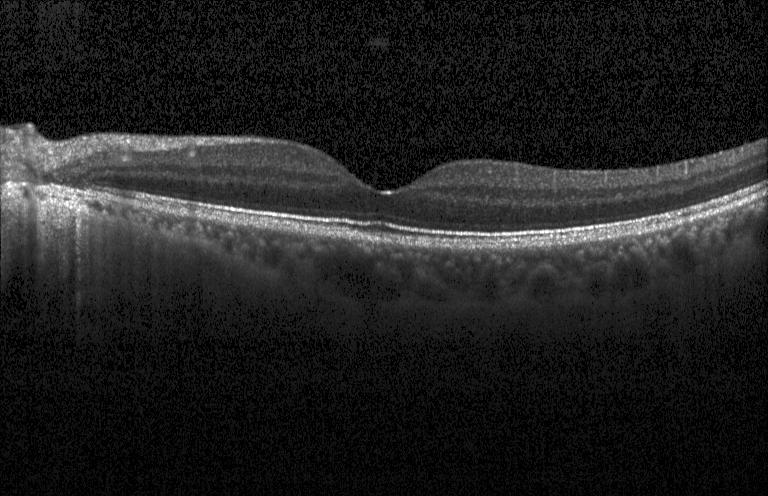
Optical coherence tomography B-scan — This B-scan demonstrates neither choroidal neovascularization, diabetic macular edema, nor drusen.